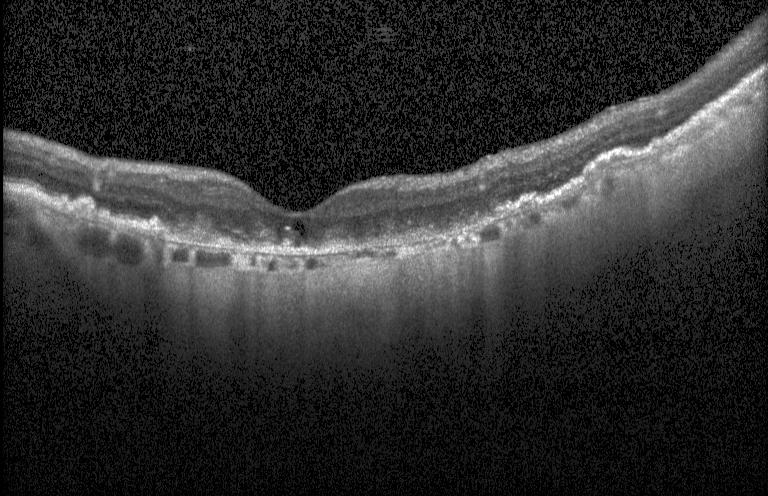 Heidelberg Spectralis, optical coherence tomography scan, spectral-domain OCT, fovea-centered. Finding: choroidal neovascularization (CNV).